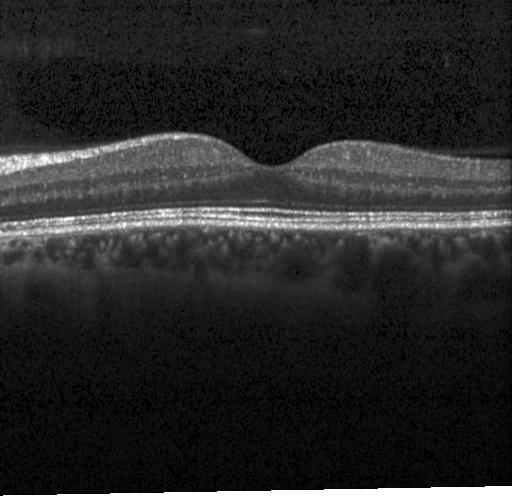
Optical coherence tomography B-scan. Horizontal scan through the fovea. Heidelberg Spectralis OCT system
Diagnosis: no evidence of choroidal neovascularization, diabetic macular edema, or drusen.